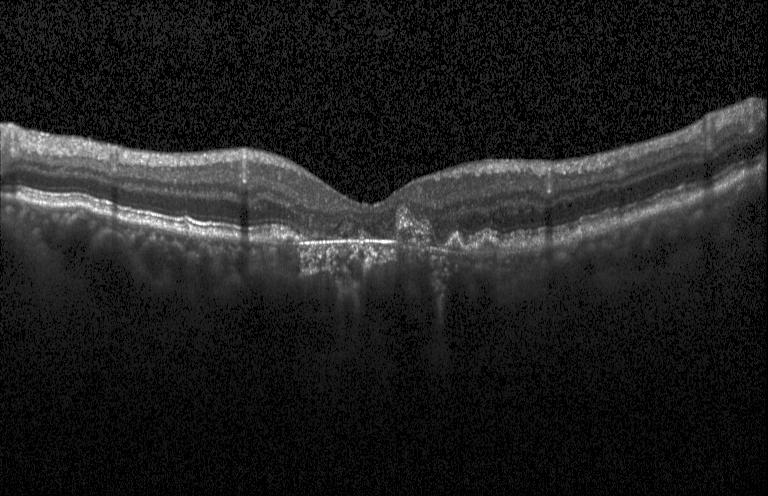
Spectral-domain OCT B-scan: a choroidal neovascular membrane.